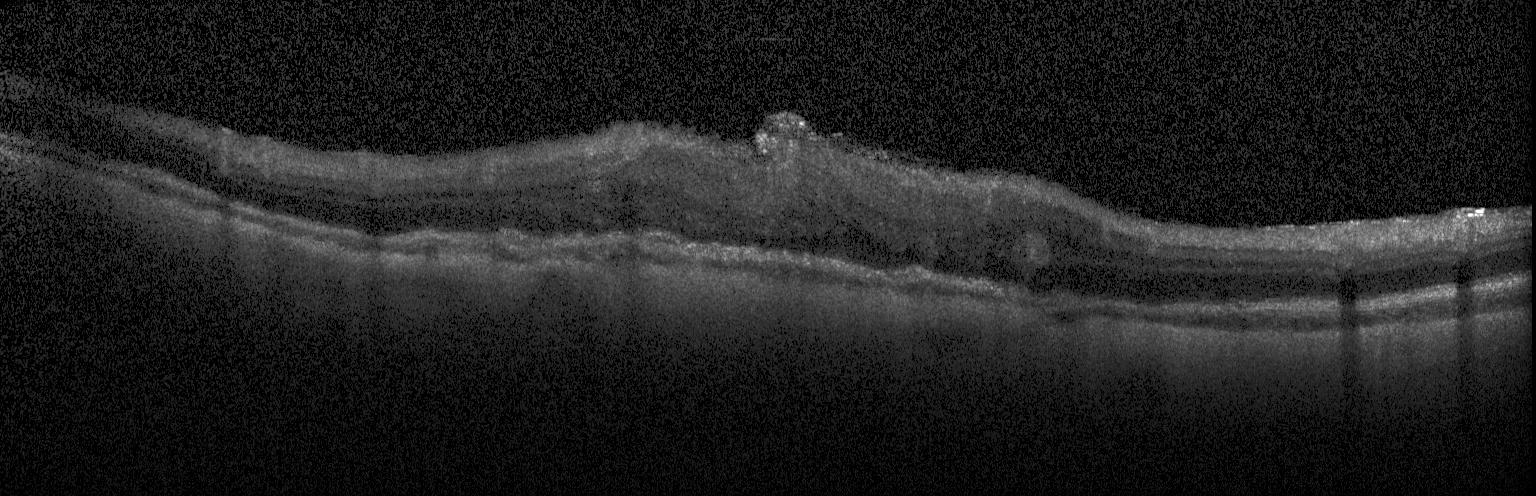
Assessment: diabetic macular edema.